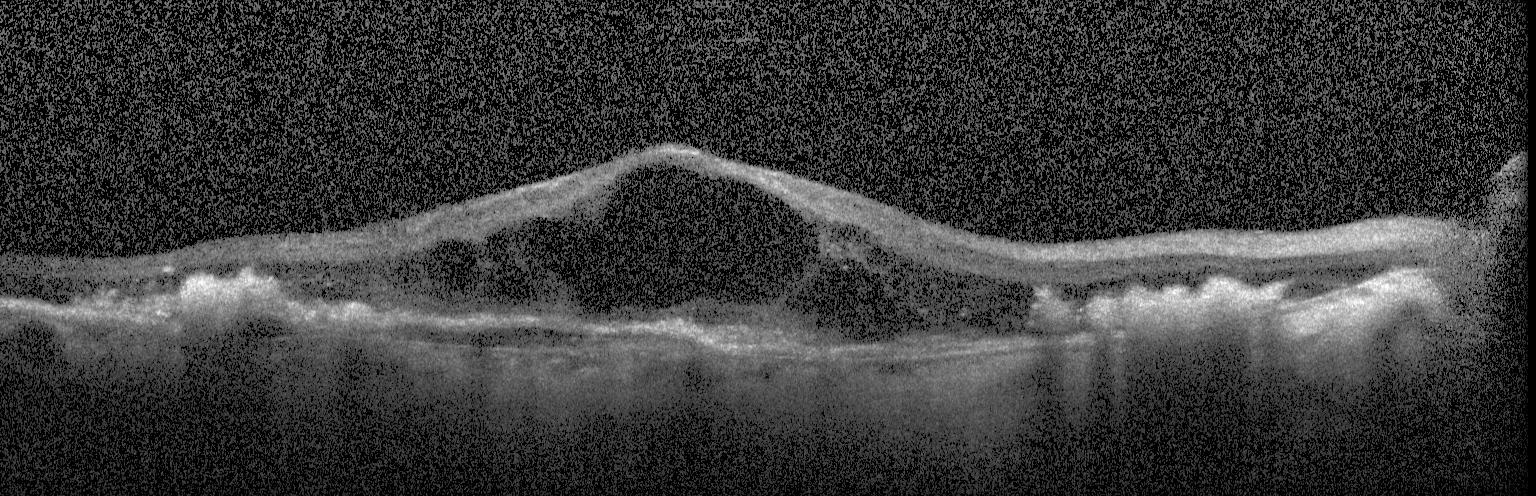 OCT finding: a choroidal neovascular membrane.